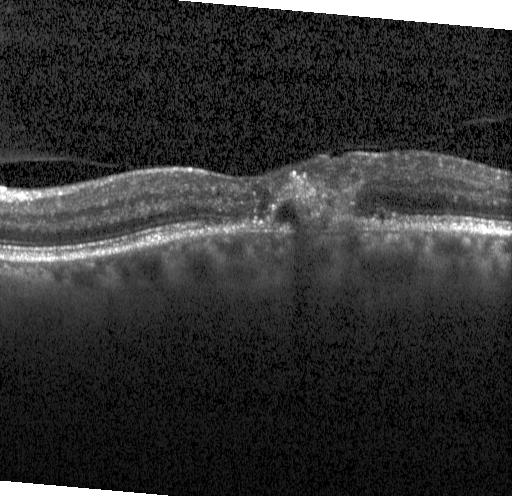 Finding: a choroidal neovascular membrane.